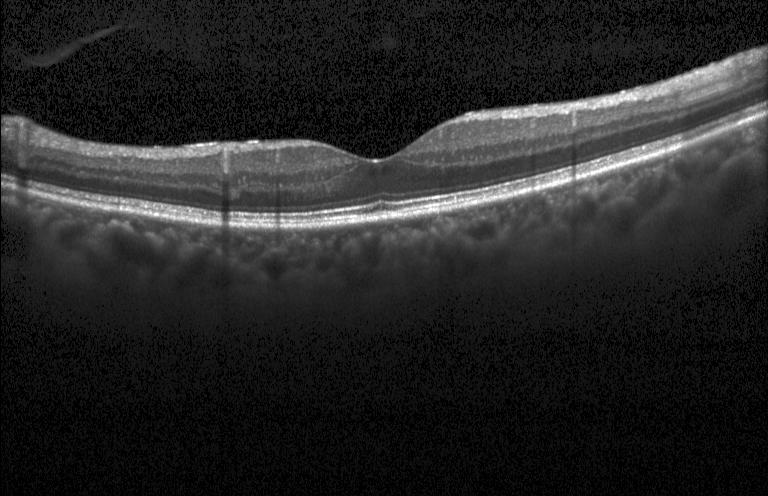

OCT B-scan.
Finding: no CNV, no DME, and no drusen.